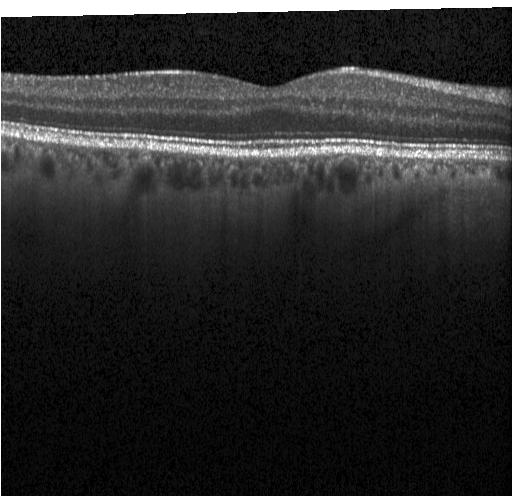 Macular scan · Heidelberg Spectralis · OCT line scan — Finding: no choroidal neovascularization, no diabetic macular edema, and no drusen.